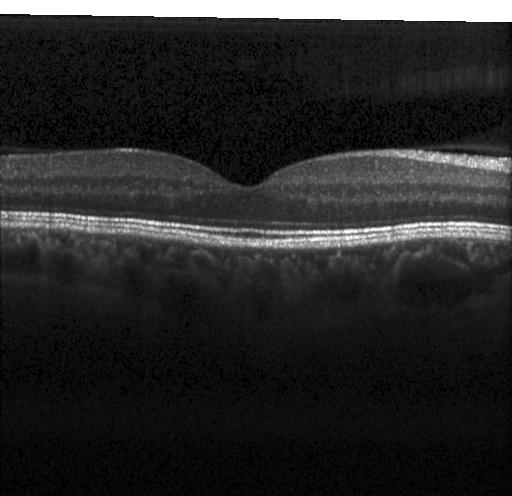
This B-scan demonstrates no evidence of choroidal neovascularization, diabetic macular edema, or drusen.